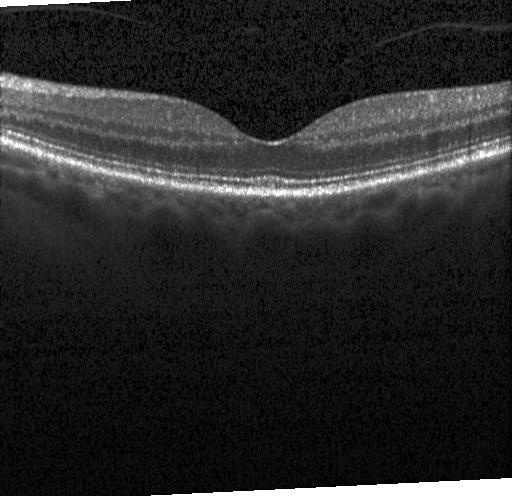 Acquired on a Heidelberg Spectralis, retinal OCT cross-section, through the macula. Finding: no evidence of choroidal neovascularization, diabetic macular edema, or drusen.